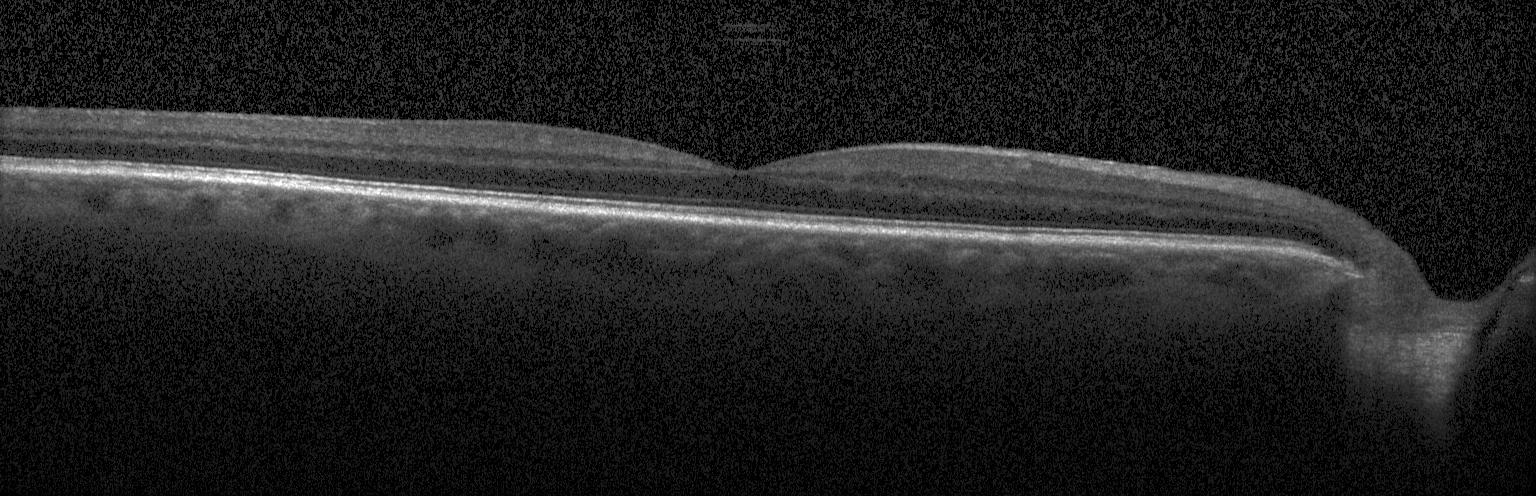
Spectral-domain OCT B-scan: no choroidal neovascularization, diabetic macular edema, or drusen.